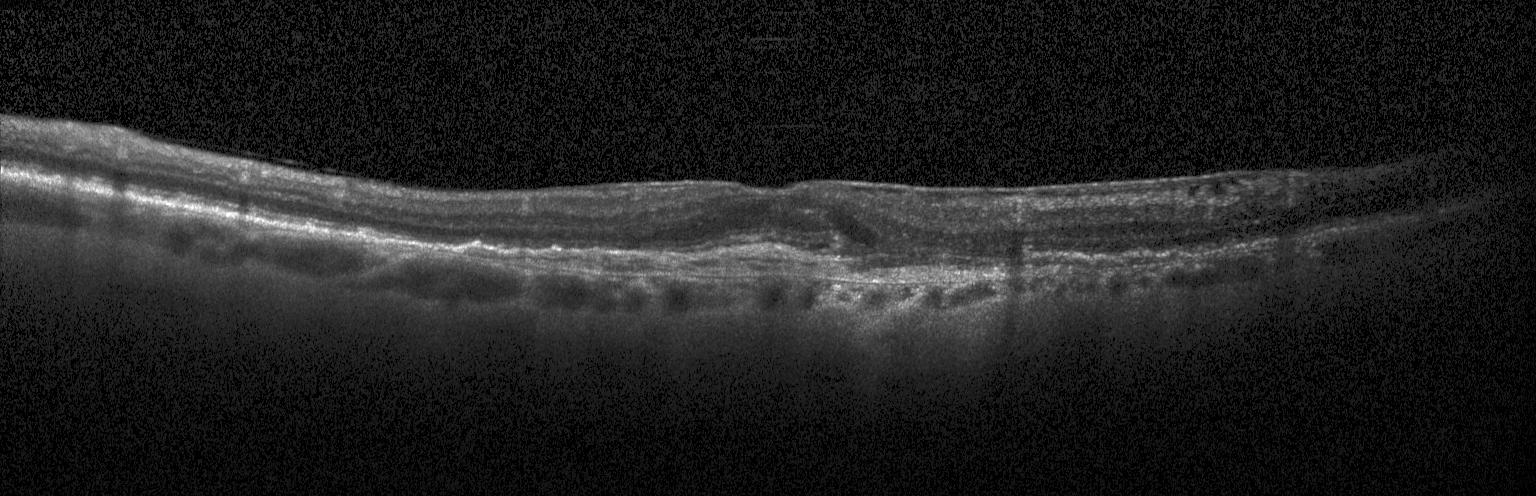 Acquired on a Heidelberg Spectralis. Optical coherence tomography scan. Horizontal scan through the fovea. CNV.